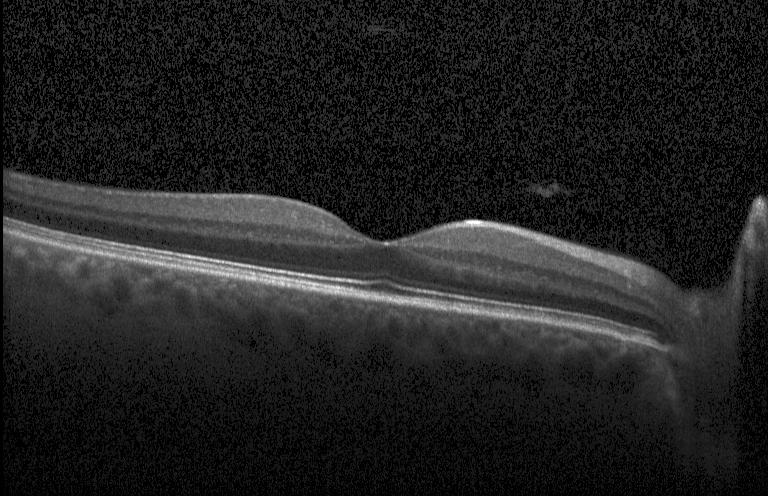

OCT B-scan; centered on the fovea
Assessment: no choroidal neovascularization, no diabetic macular edema, and no drusen.